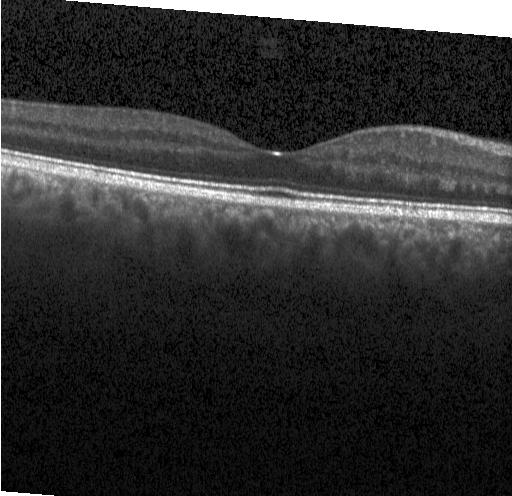
OCT scan showing no choroidal neovascularization, no diabetic macular edema, and no drusen.